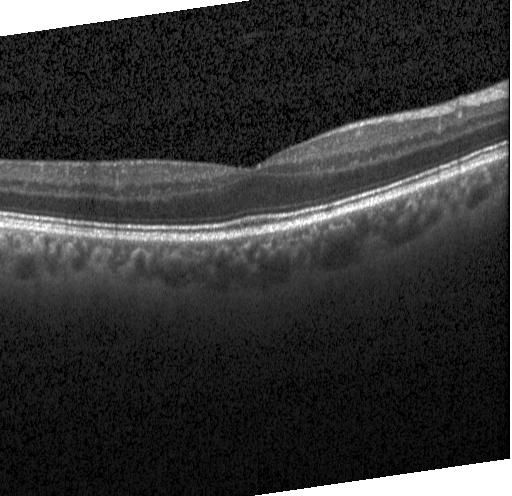

Retinal OCT cross-section.
Impression: no choroidal neovascularization, diabetic macular edema, or drusen.